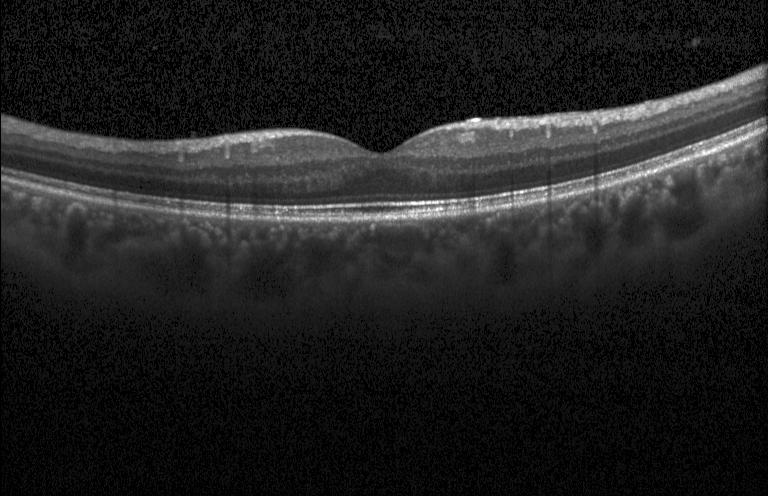

Spectral-domain optical coherence tomography · OCT line scan · through the macula · instrument: Heidelberg Spectralis — Diagnosis: no evidence of choroidal neovascularization, diabetic macular edema, or drusen.